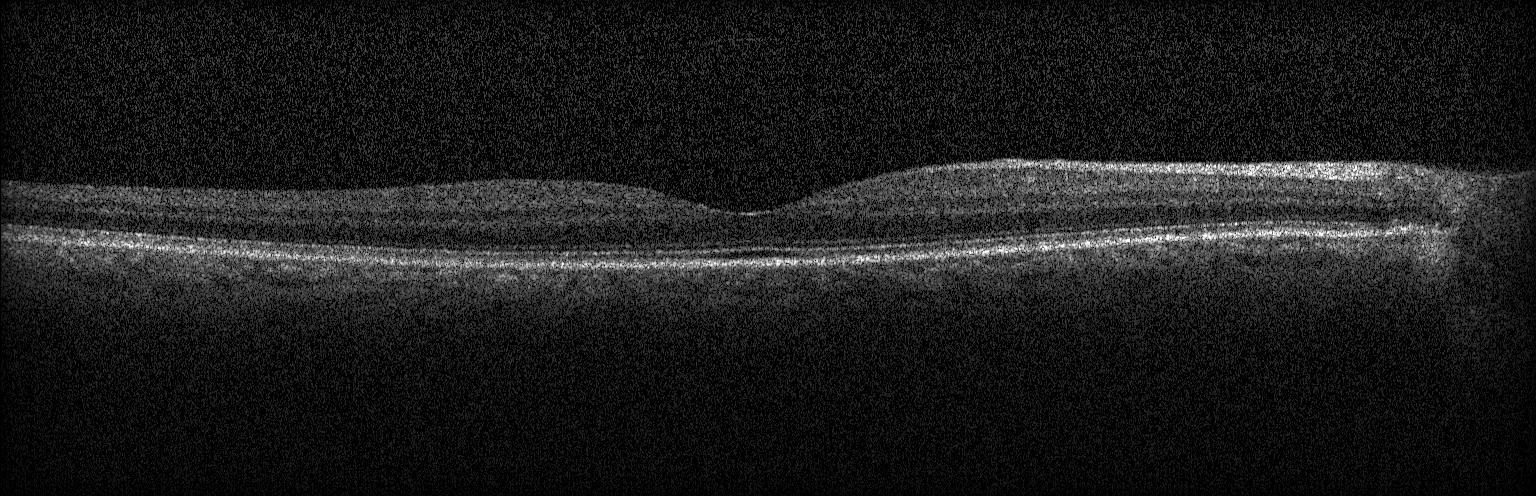

OCT B-scan — Finding: neither CNV, DME, nor drusen.